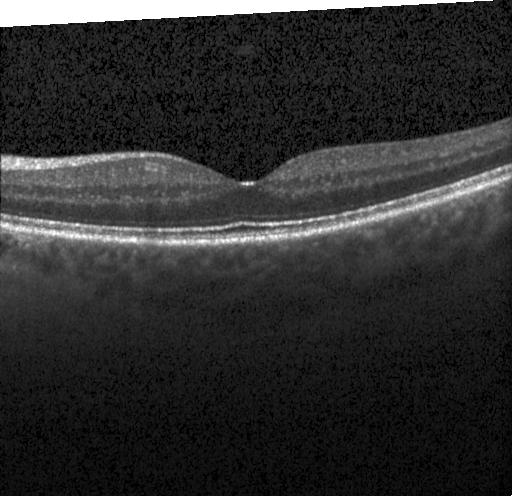 Spectral-domain optical coherence tomography; OCT B-scan.
Impression: no choroidal neovascularization, no diabetic macular edema, and no drusen.